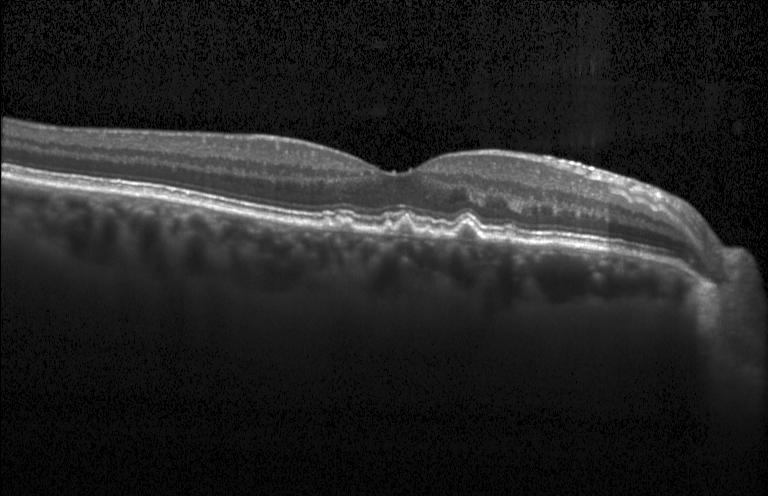 Optical coherence tomography scan, SD-OCT, centered on the fovea.
Finding: multiple drusen.